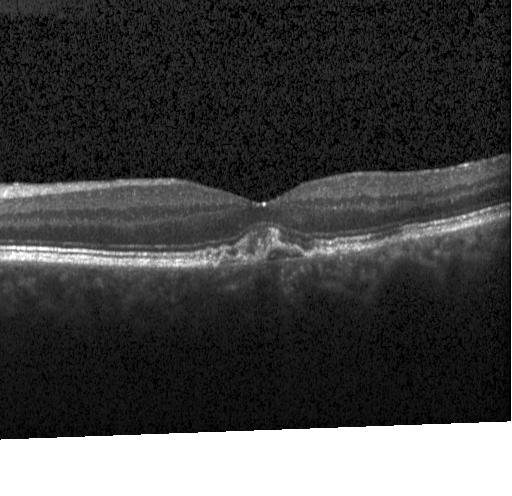 Spectral-domain OCT · macular scan · instrument: Heidelberg Spectralis · optical coherence tomography scan
A choroidal neovascular membrane.